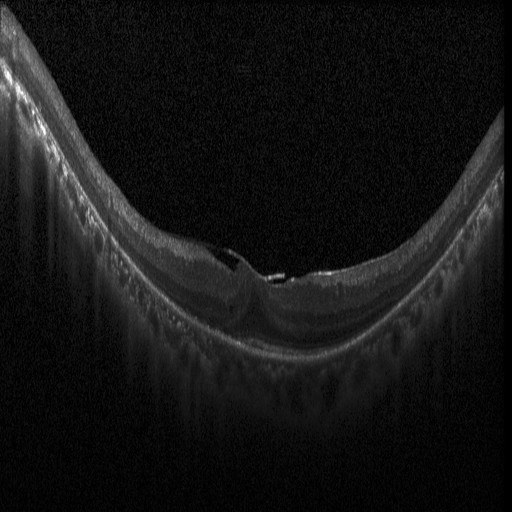 Heidelberg Spectralis OCT system, retinal OCT cross-section, spectral-domain optical coherence tomography.
This B-scan demonstrates diabetic macular edema (DME).